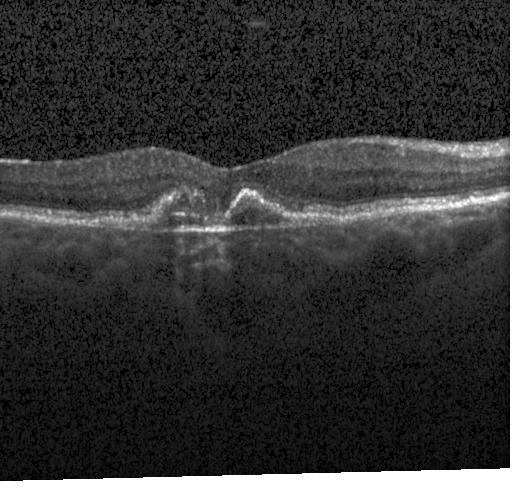

Optical coherence tomography B-scan, fovea-centered, spectral-domain optical coherence tomography, instrument: Heidelberg Spectralis.
Diagnosis: choroidal neovascularization.